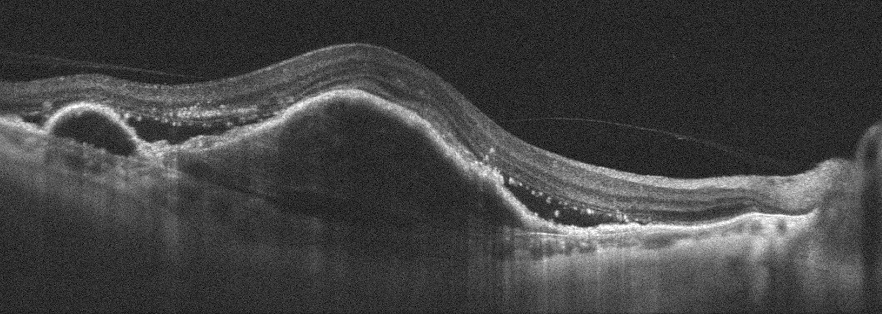 Impression: age-related macular degeneration.